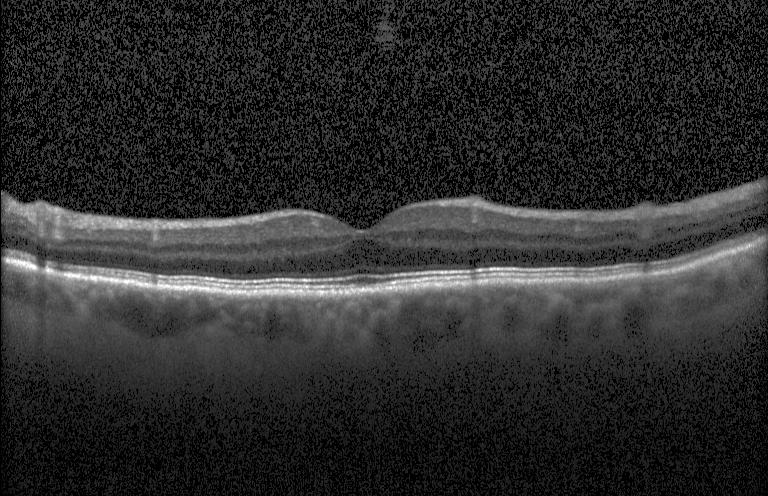

Through the macula; retinal OCT cross-section; instrument: Heidelberg Spectralis.
OCT finding: no choroidal neovascularization, no diabetic macular edema, and no drusen.